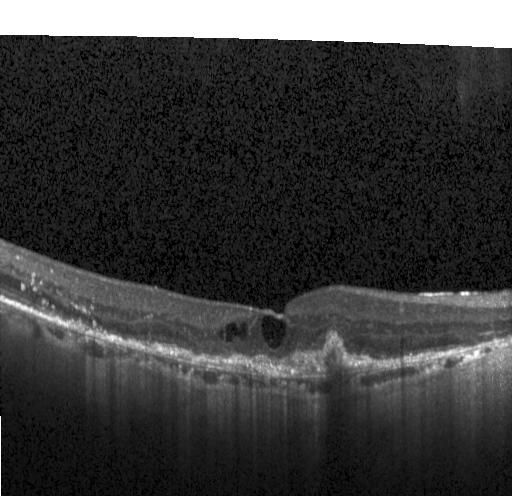

OCT scan showing a choroidal neovascular membrane.